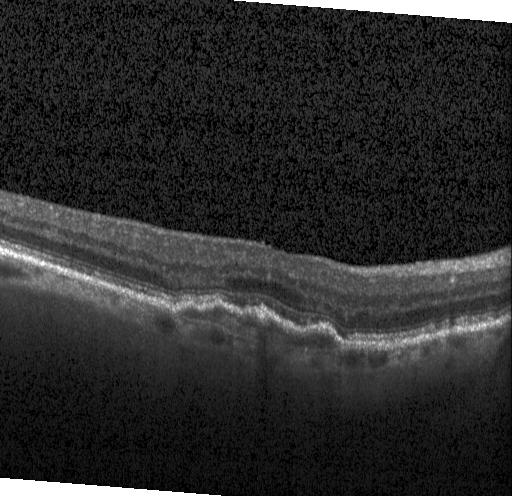
Through the macula, retinal OCT B-scan, acquired on a Heidelberg Spectralis
The scan shows a choroidal neovascular membrane.